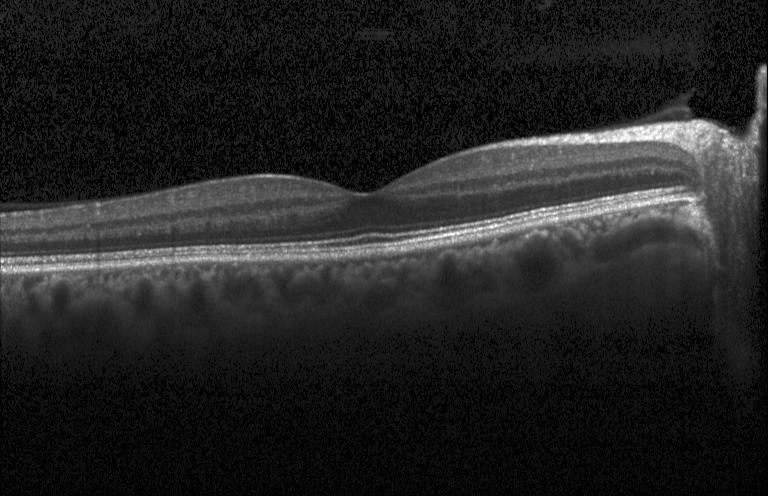

Optical coherence tomography B-scan — Diagnosis: no CNV, no DME, and no drusen.